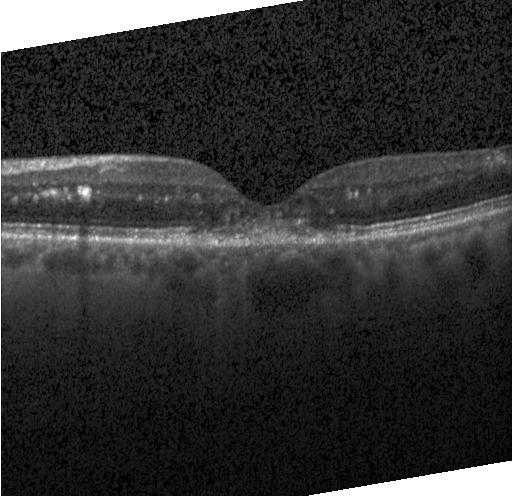 OCT B-scan showing choroidal neovascularization.